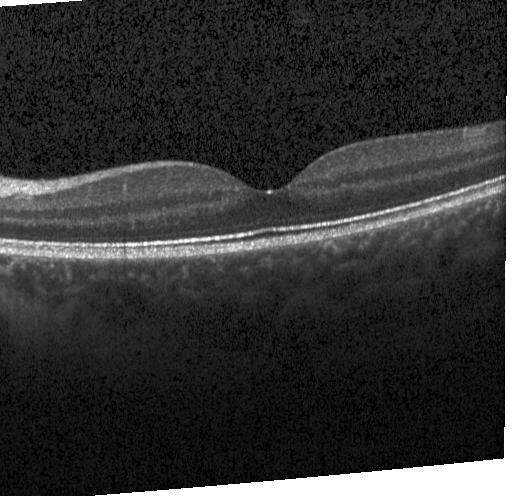
Dx: no choroidal neovascularization, no diabetic macular edema, and no drusen.